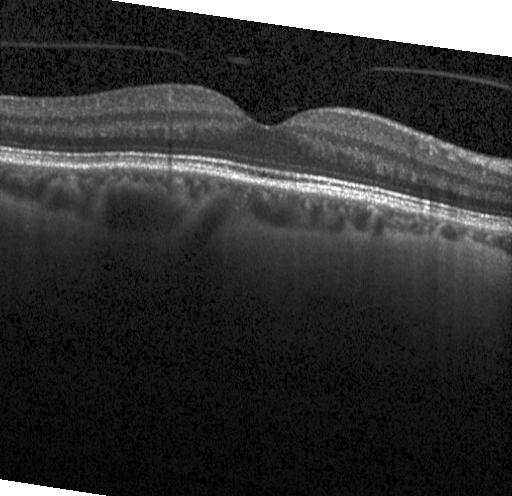

OCT B-scan.
Assessment: no evidence of CNV, DME, or drusen.